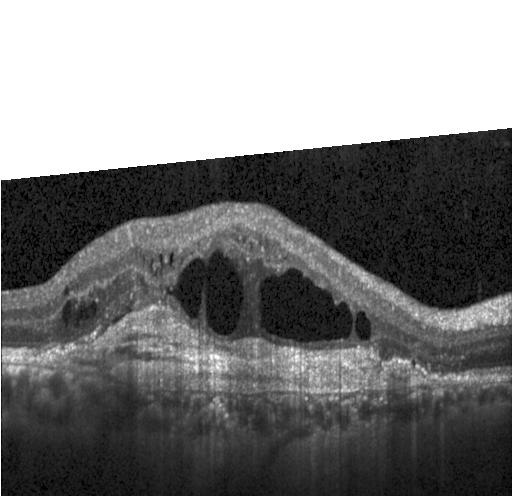
OCT B-scan; spectral-domain OCT; fovea-centered.
Finding: CNV.